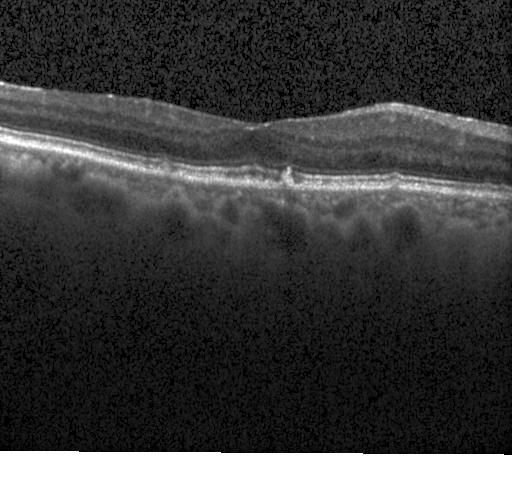

Optical coherence tomography scan · instrument: Heidelberg Spectralis
Diagnosis: multiple drusen.